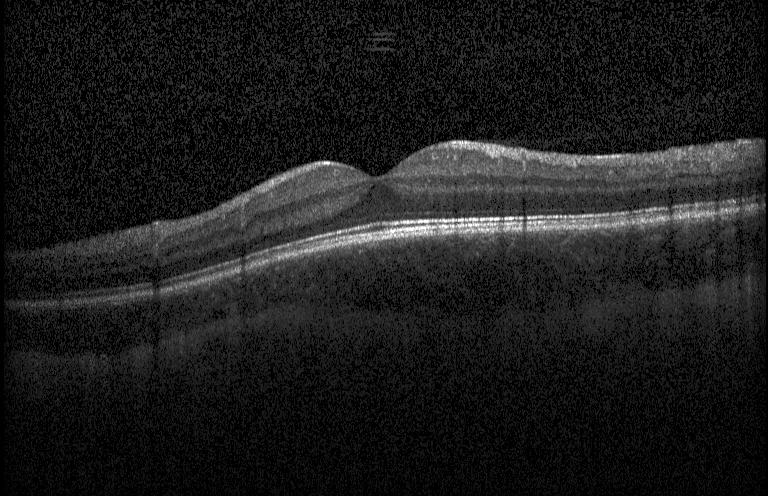
Macular OCT: neither choroidal neovascularization, diabetic macular edema, nor drusen.